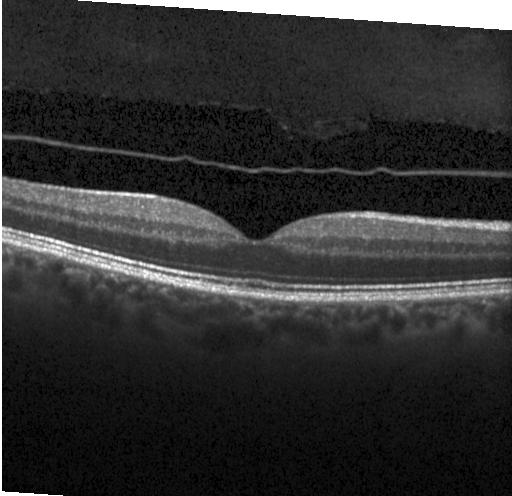 Macular OCT: no choroidal neovascularization, no diabetic macular edema, and no drusen.